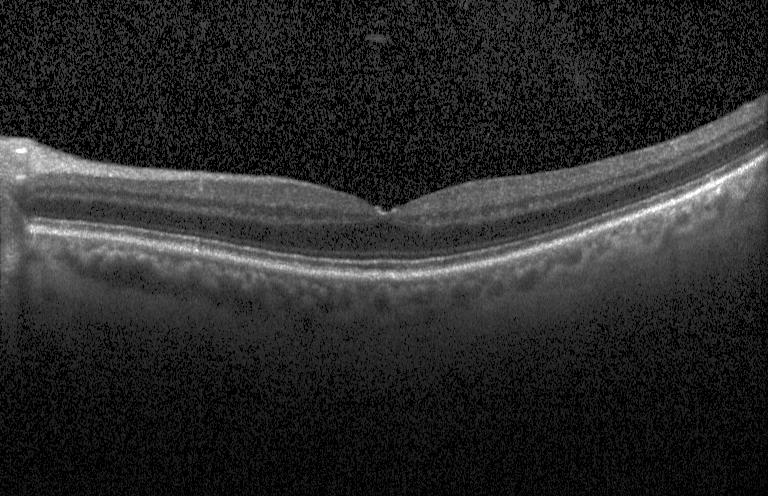
Spectral-domain OCT · macular scan · instrument: Heidelberg Spectralis · OCT B-scan
Diagnosis: no choroidal neovascularization, no diabetic macular edema, and no drusen.